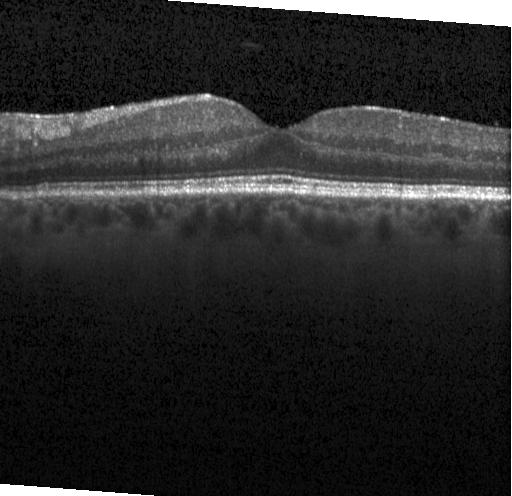

OCT B-scan. Macular scan. Spectral-domain optical coherence tomography. Heidelberg Spectralis — Assessment: no CNV, DME, or drusen.